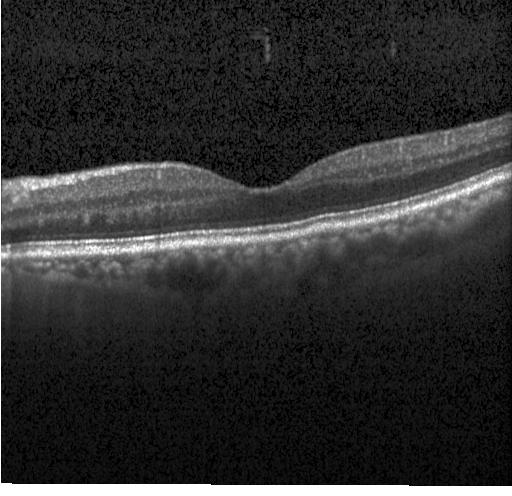 Dx: no CNV, DME, or drusen.